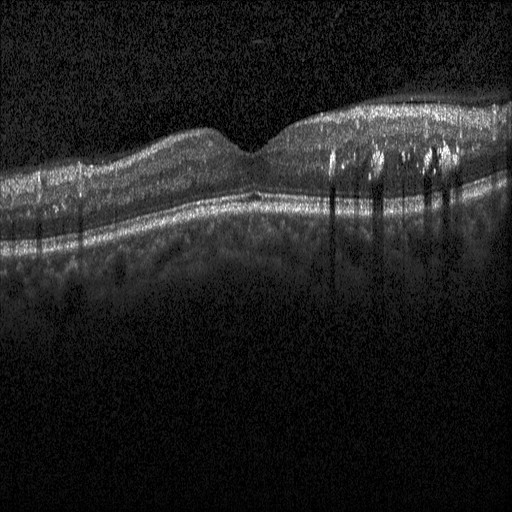 OCT B-scan showing diabetic macular edema.